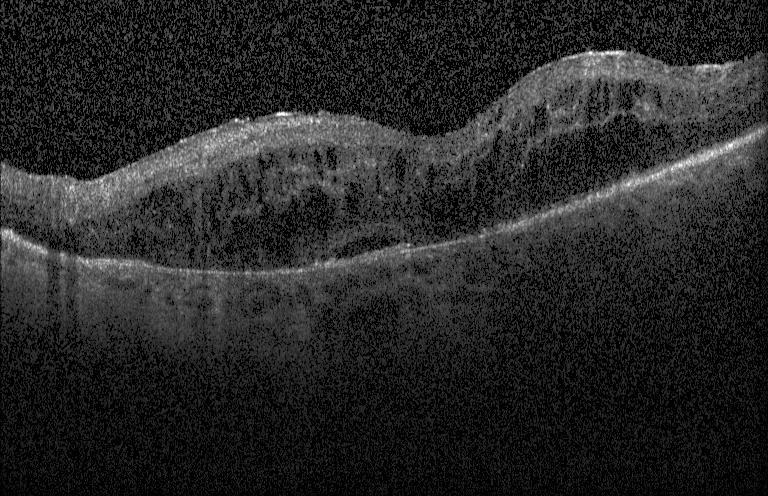
OCT scan showing choroidal neovascularization (CNV).